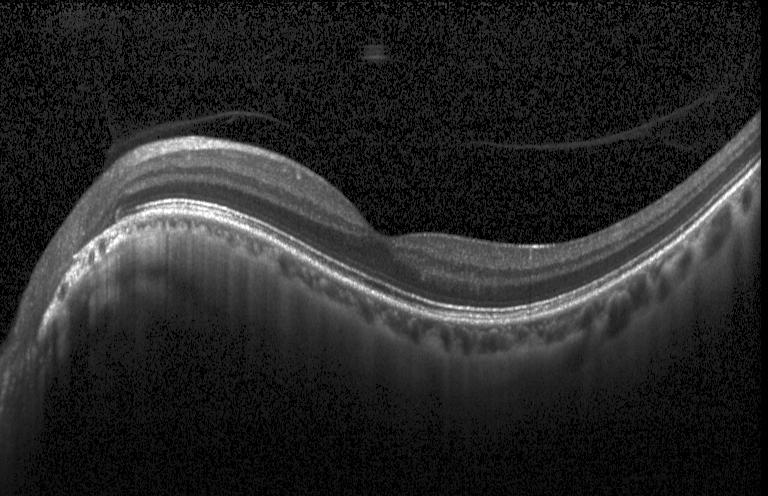

The scan shows no choroidal neovascularization, diabetic macular edema, or drusen.